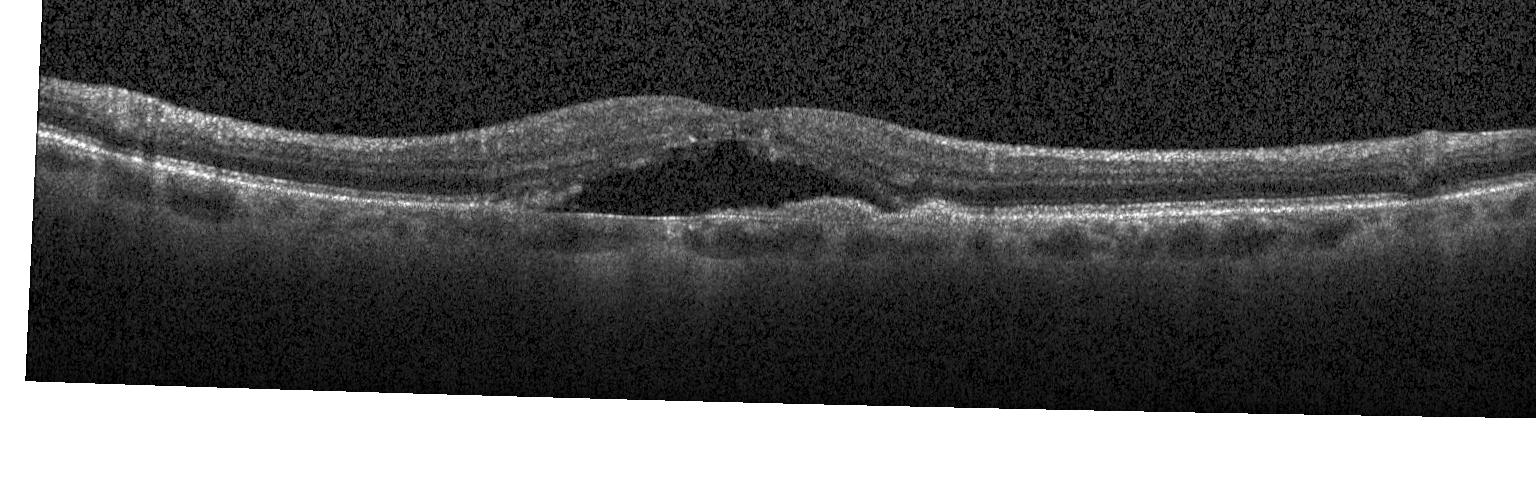

Impression: CNV.